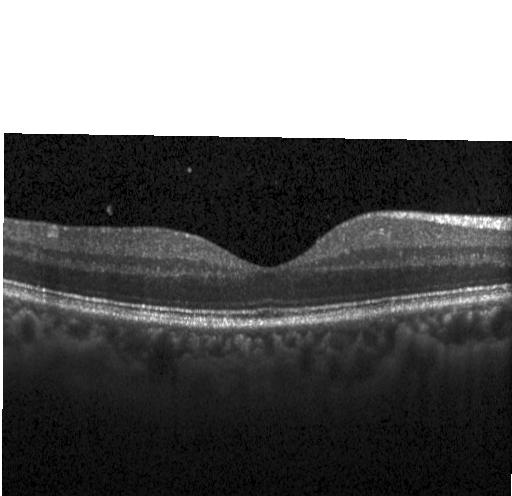 Retinal OCT B-scan.
Diagnosis: no evidence of choroidal neovascularization, diabetic macular edema, or drusen.